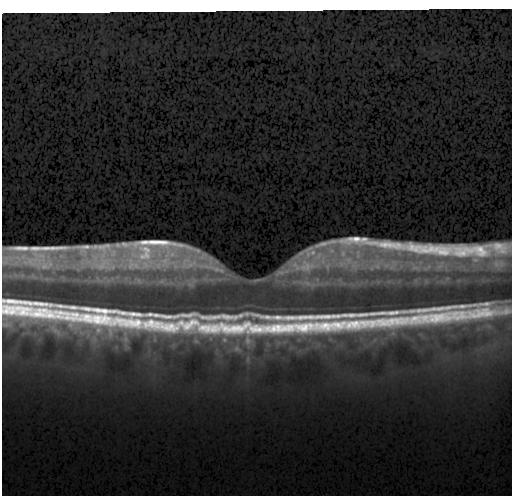

Diagnosis: drusen.